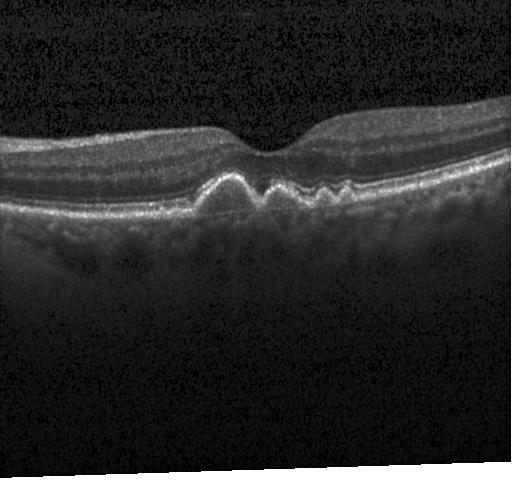 OCT scan showing sub-RPE drusenoid deposits.